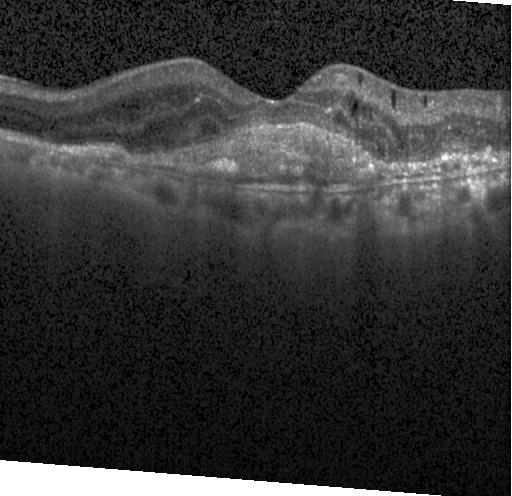

Diagnosis: choroidal neovascularization.